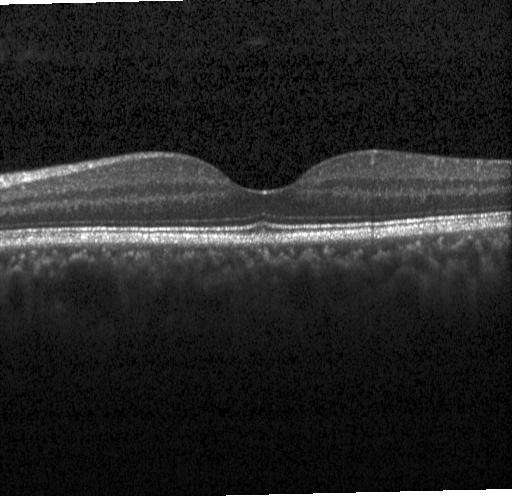 Retinal OCT cross-section showing no choroidal neovascularization, no diabetic macular edema, and no drusen.